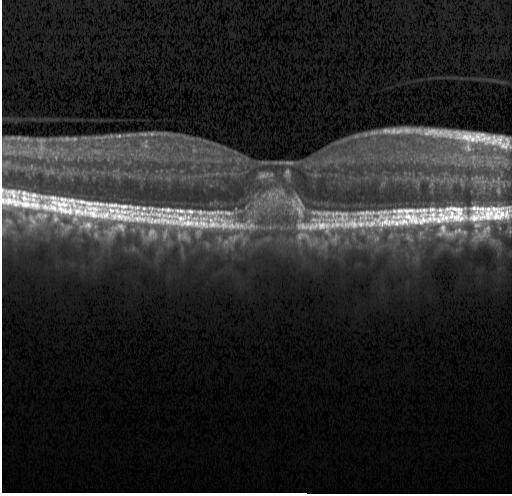

OCT line scan. Macular scan
Impression: a choroidal neovascular membrane.